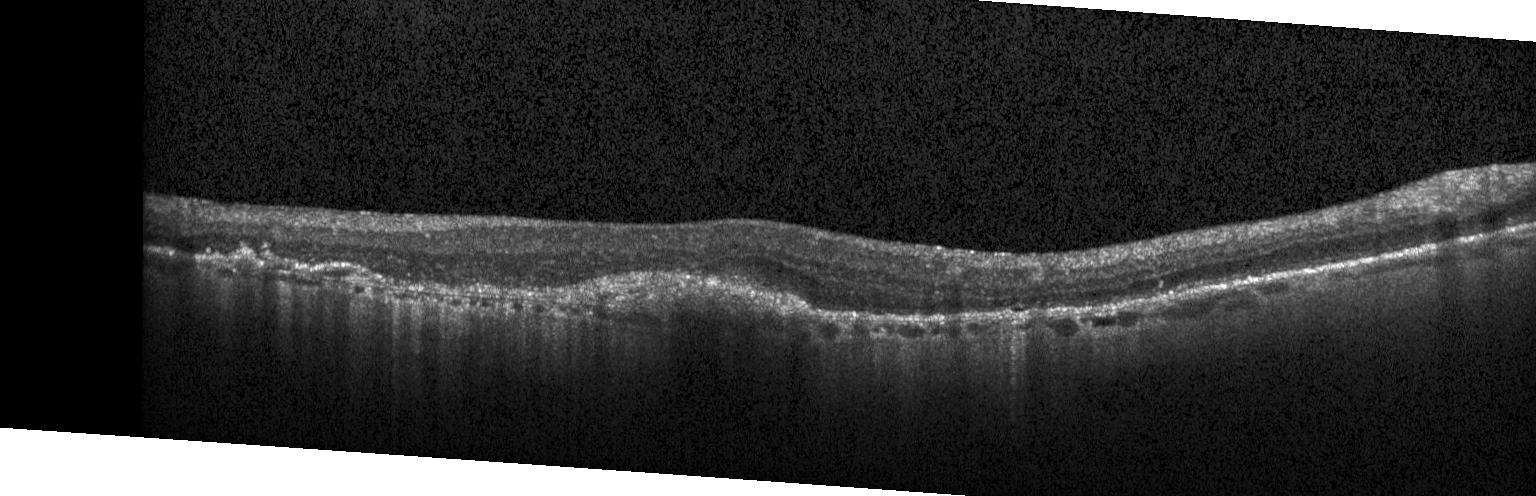 Retinal OCT cross-section. Impression: a choroidal neovascular membrane.